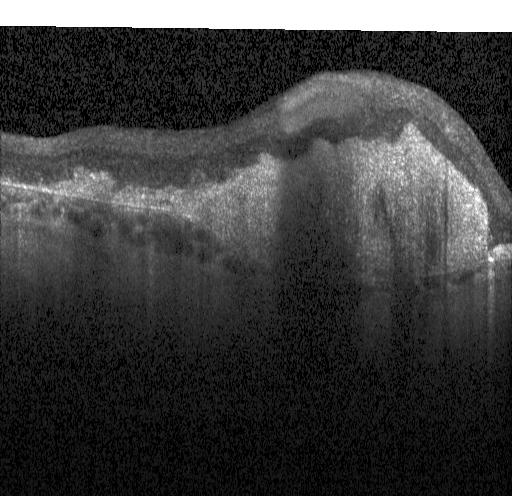

Finding: choroidal neovascularization.